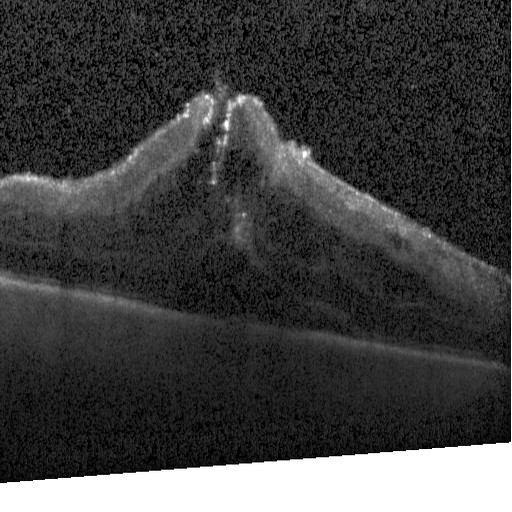 Retinal OCT B-scan. Diagnosis: DME.